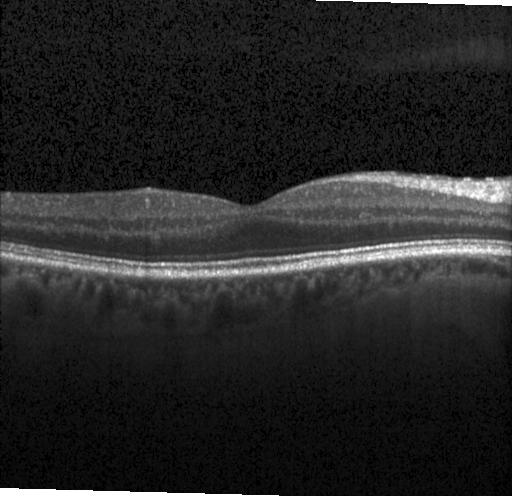

OCT B-scan — Assessment: neither choroidal neovascularization, diabetic macular edema, nor drusen.